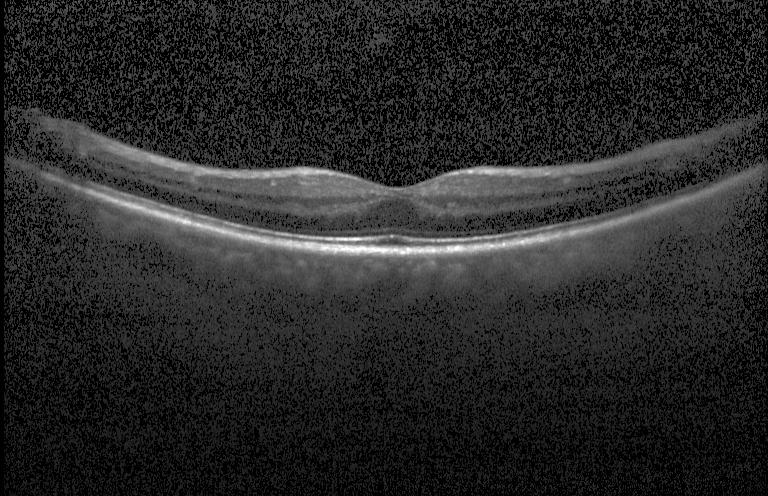
OCT scan showing no choroidal neovascularization, diabetic macular edema, or drusen.